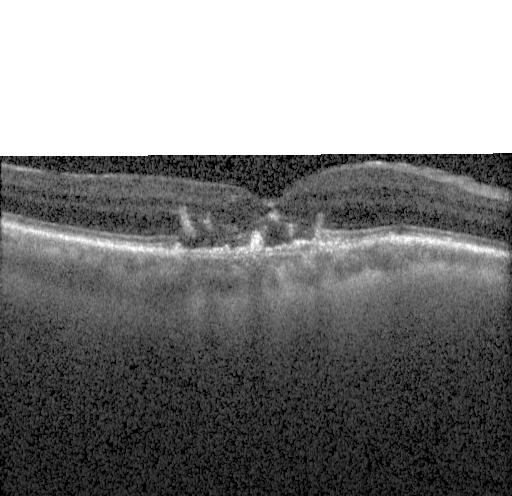

Assessment: a choroidal neovascular membrane.